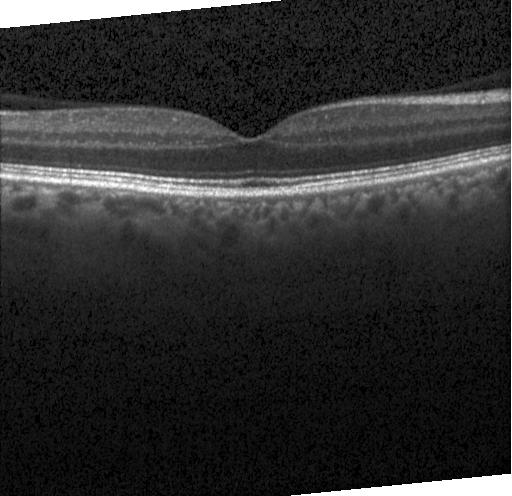

Finding: no CNV, DME, or drusen.